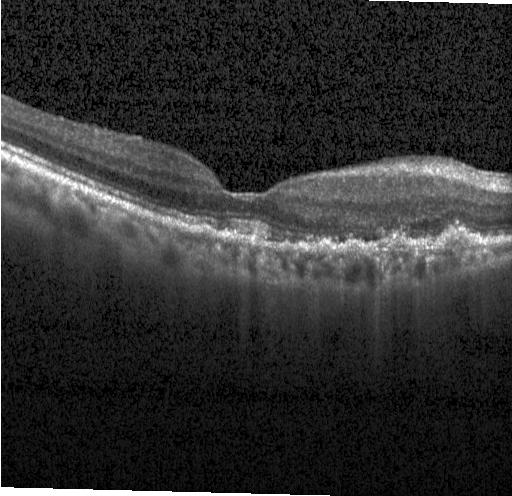 Retinal OCT cross-section, centered on the fovea.
A choroidal neovascular membrane.